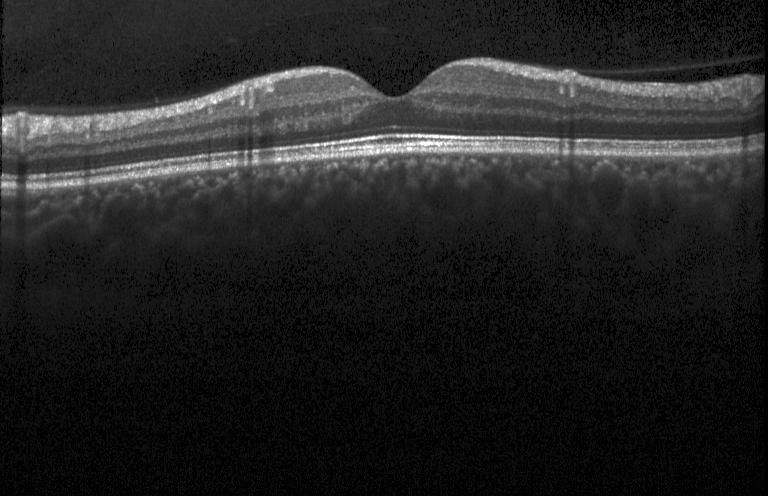

Centered on the fovea, spectral-domain optical coherence tomography, acquired on a Heidelberg Spectralis, OCT line scan — This B-scan demonstrates neither choroidal neovascularization, diabetic macular edema, nor drusen.